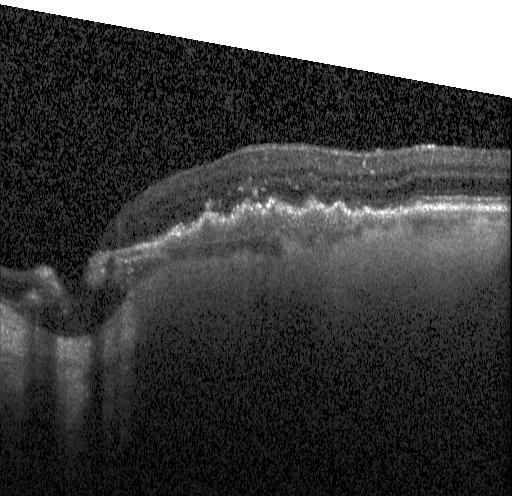
Finding: choroidal neovascularization.